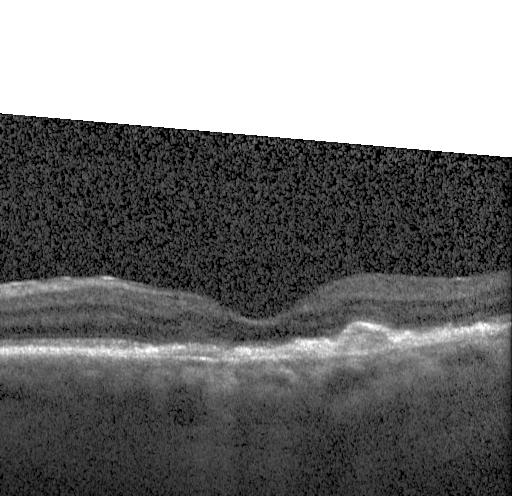

The scan shows a choroidal neovascular membrane.